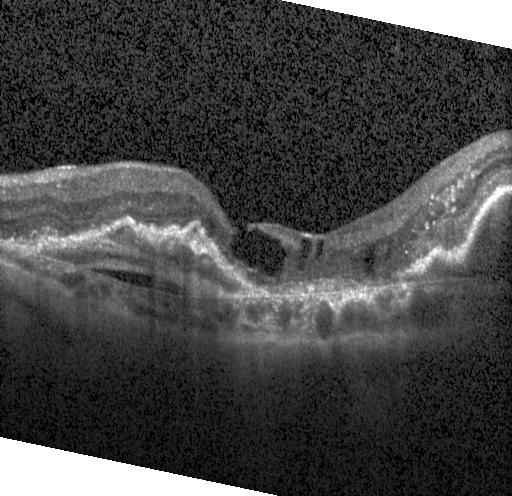

Dx: a choroidal neovascular membrane.